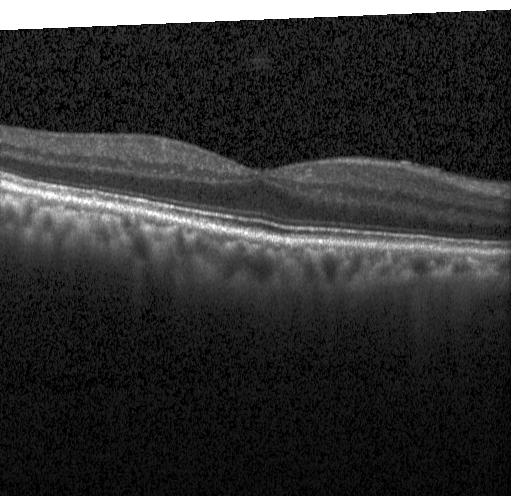
Retinal OCT cross-section
Dx: no choroidal neovascularization, no diabetic macular edema, and no drusen.